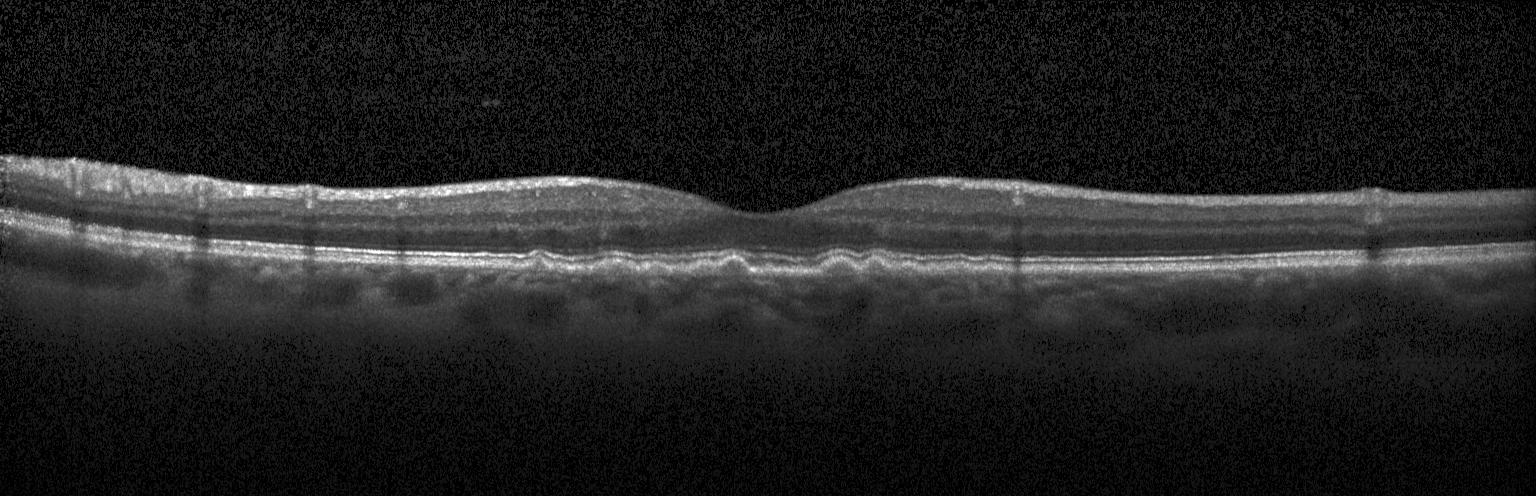

Spectral-domain OCT · OCT B-scan — Finding: multiple drusen.